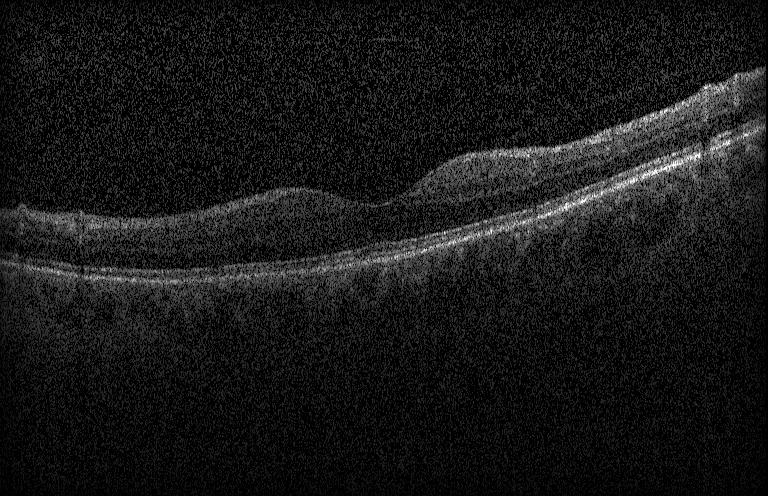
Retinal OCT B-scan. This B-scan demonstrates no choroidal neovascularization, diabetic macular edema, or drusen.